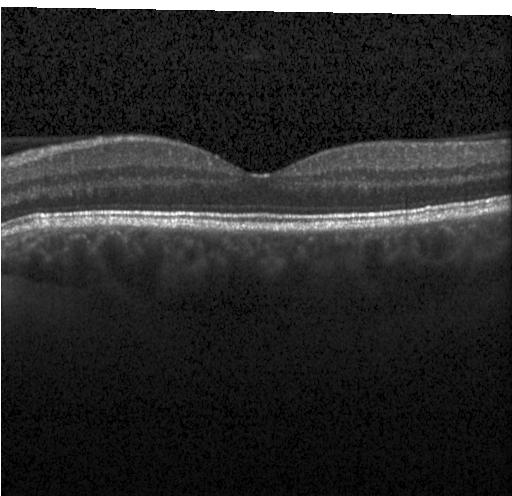 The scan shows no evidence of choroidal neovascularization, diabetic macular edema, or drusen.